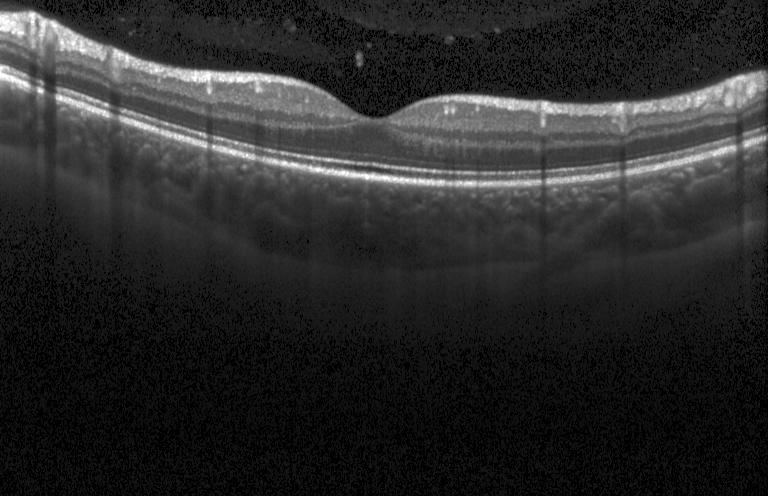
Spectral-domain optical coherence tomography · optical coherence tomography B-scan · centered on the fovea · instrument: Heidelberg Spectralis — Diagnosis: no evidence of choroidal neovascularization, diabetic macular edema, or drusen.